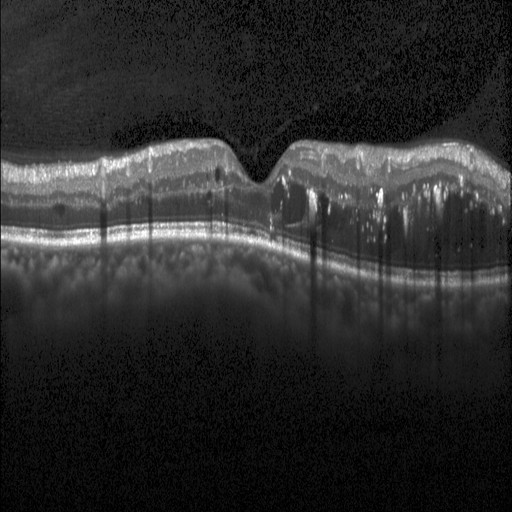 OCT B-scan.
This B-scan demonstrates diabetic macular edema (DME).